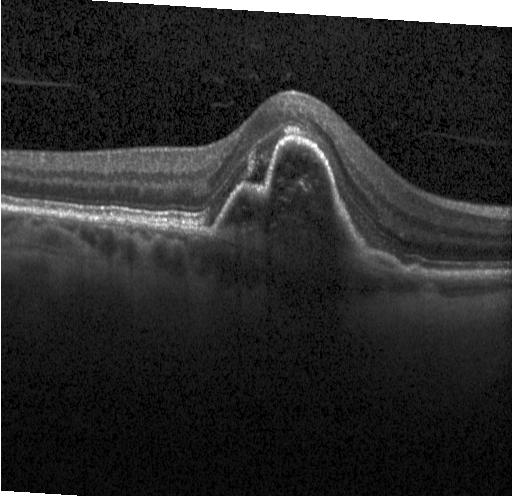
Macular scan; retinal OCT cross-section; spectral-domain optical coherence tomography. This B-scan demonstrates a choroidal neovascular membrane.